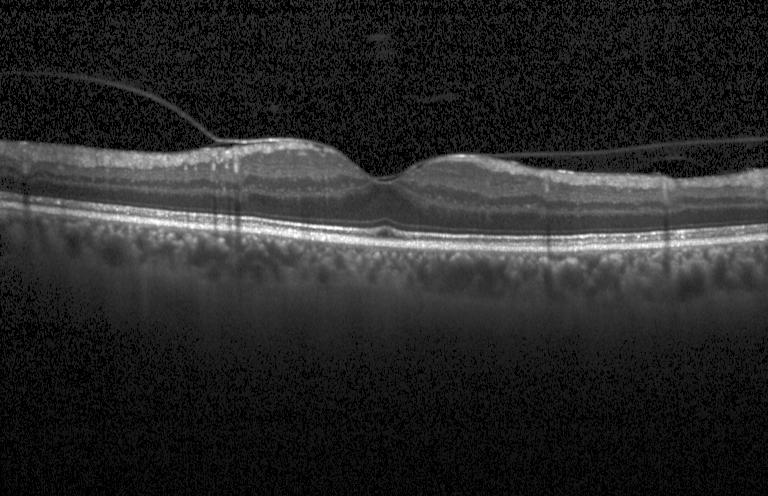
OCT B-scan, spectral-domain optical coherence tomography — Diagnosis: no CNV, DME, or drusen.